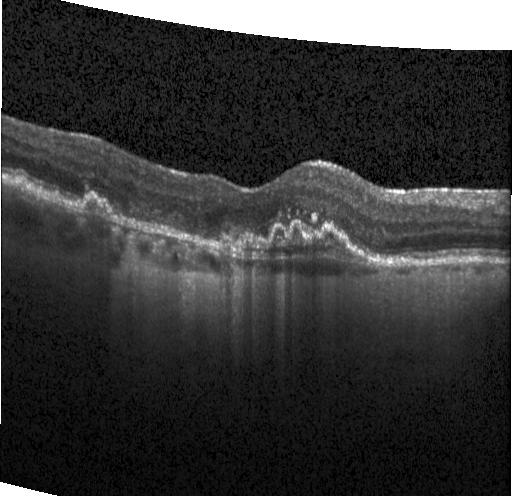
Centered on the fovea. Optical coherence tomography B-scan. Spectral-domain OCT.
This B-scan demonstrates a choroidal neovascular membrane.